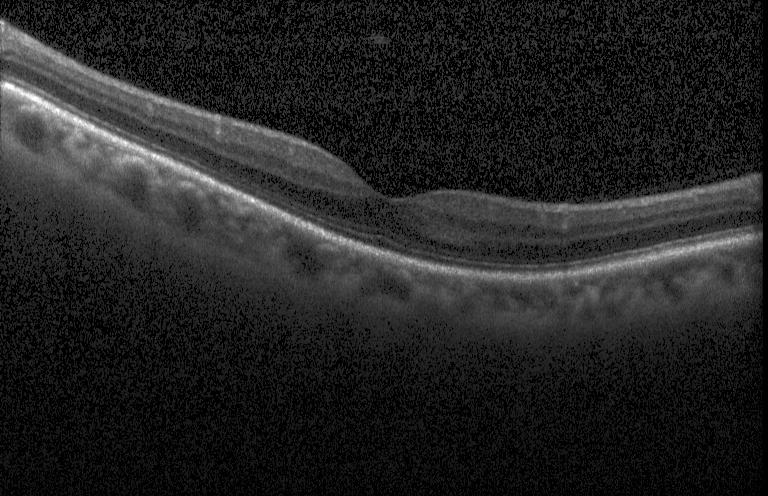

Dx: no CNV, no DME, and no drusen.